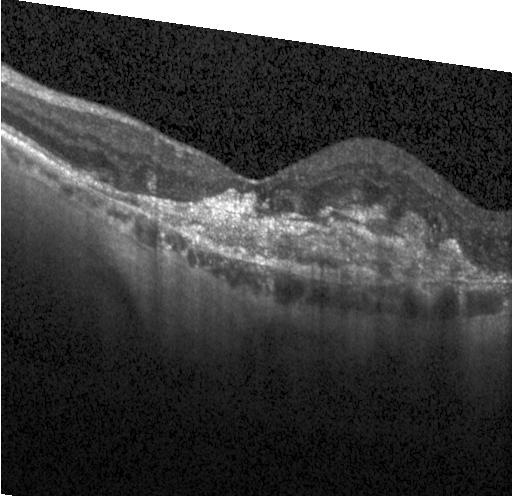

Finding: a choroidal neovascular membrane.